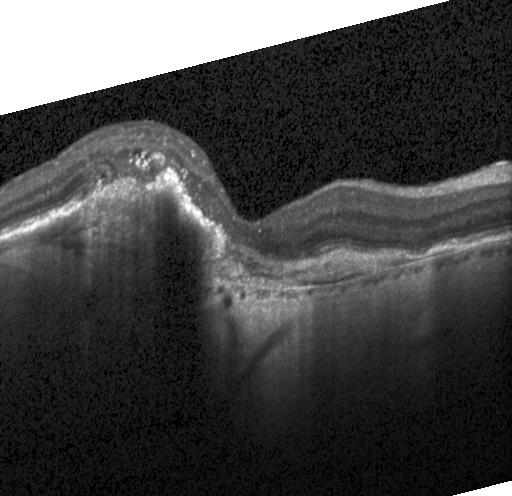

Retinal OCT B-scan
Impression: a choroidal neovascular membrane.